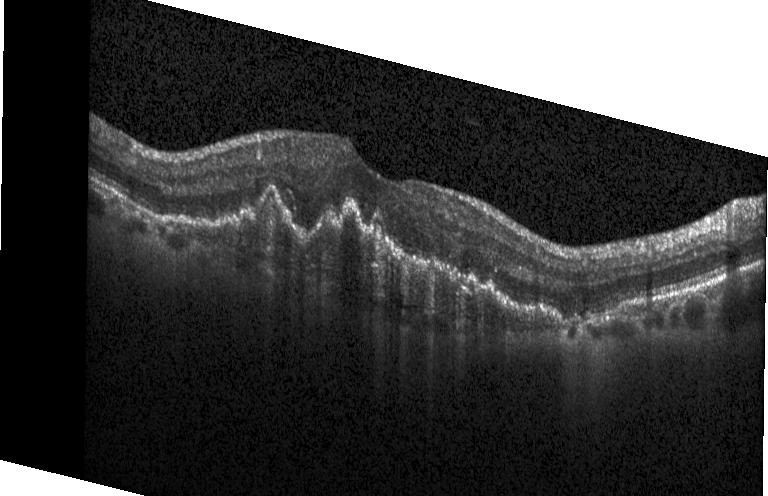
Instrument: Heidelberg Spectralis; optical coherence tomography B-scan; spectral-domain OCT; through the macula.
Impression: a choroidal neovascular membrane.